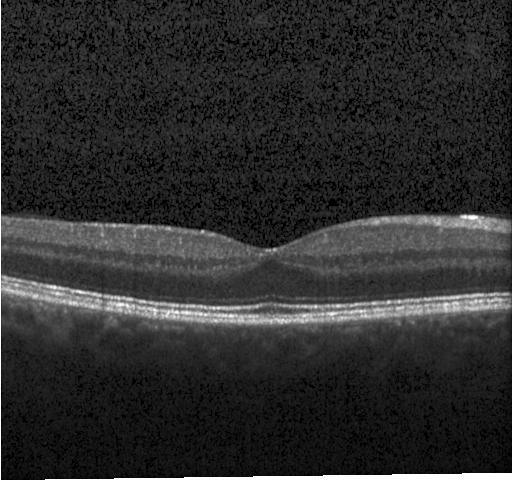

Heidelberg Spectralis OCT system, OCT B-scan, spectral-domain OCT.
Dx: no evidence of choroidal neovascularization, diabetic macular edema, or drusen.